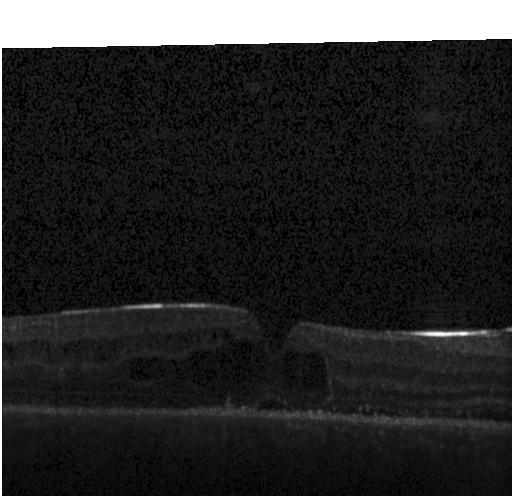

Spectral-domain OCT; acquired on a Heidelberg Spectralis; OCT B-scan; fovea-centered — Impression: diabetic macular edema (DME).